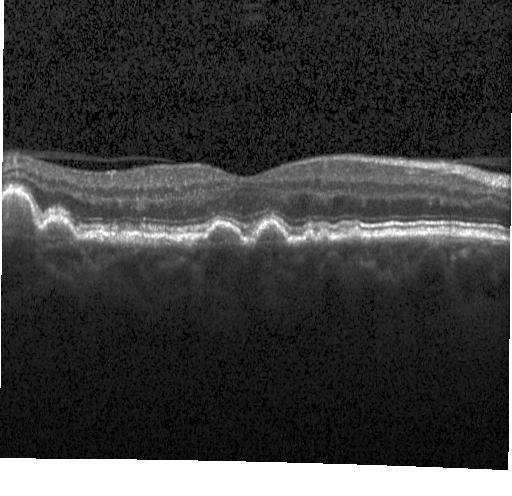

Horizontal scan through the fovea · retinal OCT cross-section · spectral-domain OCT
Impression: drusen.